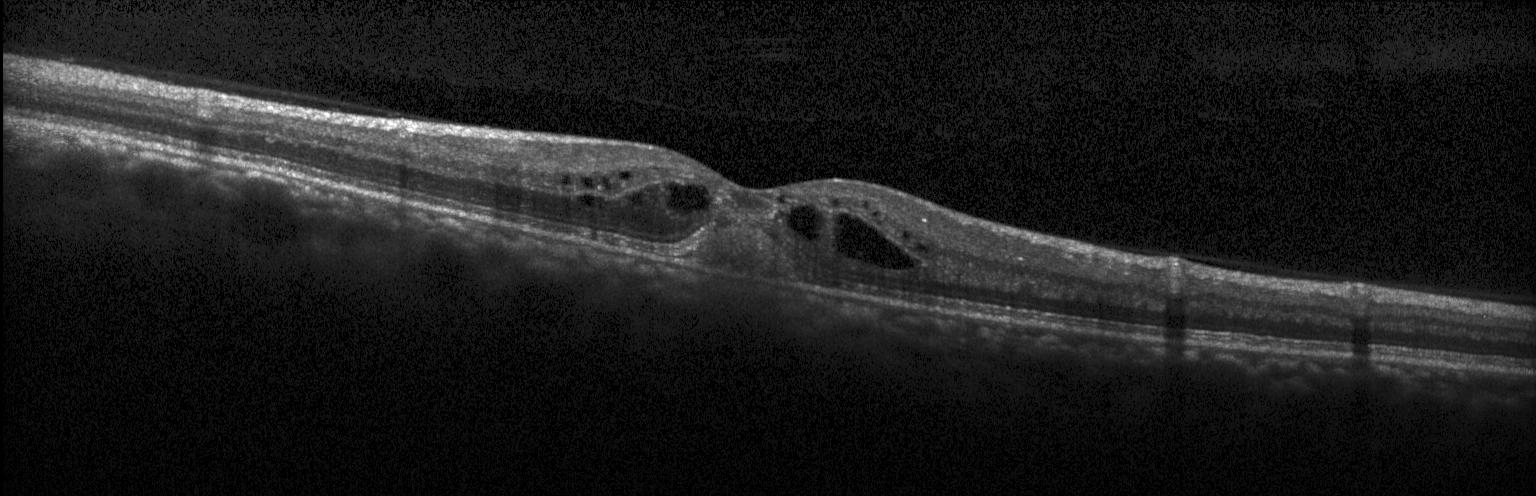

Assessment: choroidal neovascularization (CNV).